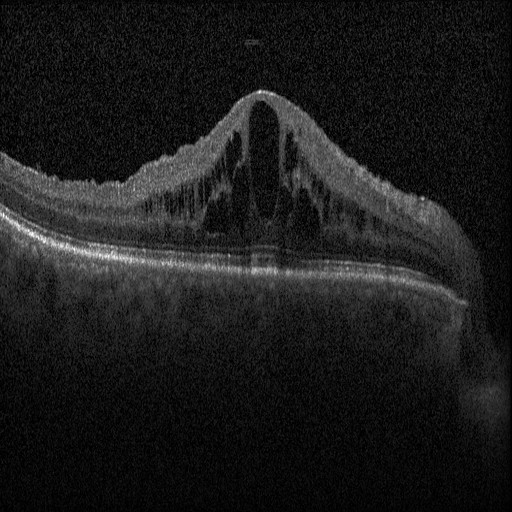 Macular OCT: diabetic macular edema (DME).